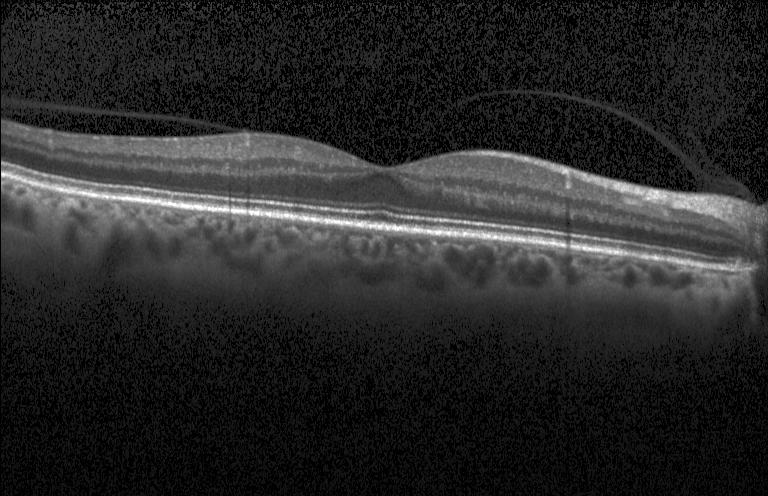 Macular OCT: no CNV, no DME, and no drusen.